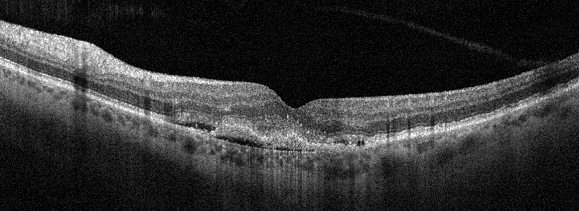 OS, fovea-centered, retinal OCT cross-section, instrument: Optovue Avanti RTVue XR.
Diagnosis: age-related macular degeneration.